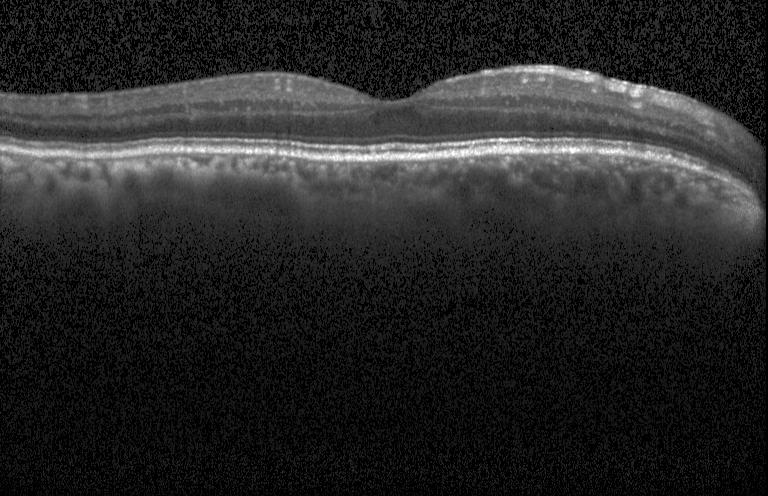
Retinal OCT B-scan — Macular OCT: neither choroidal neovascularization, diabetic macular edema, nor drusen.